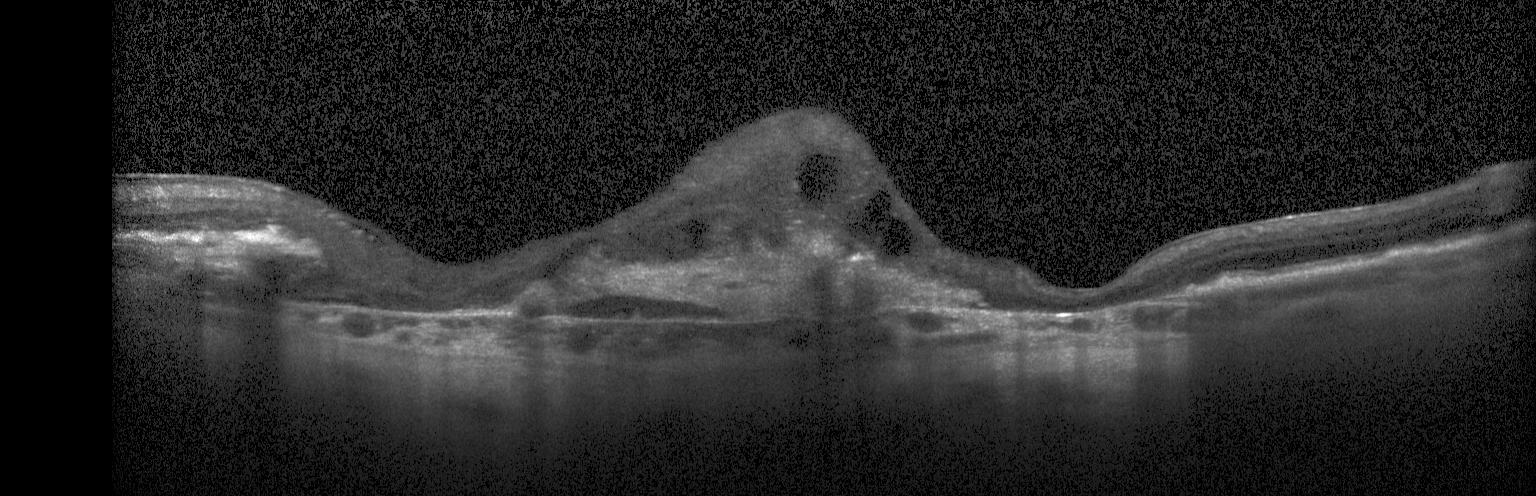 Assessment: a choroidal neovascular membrane.